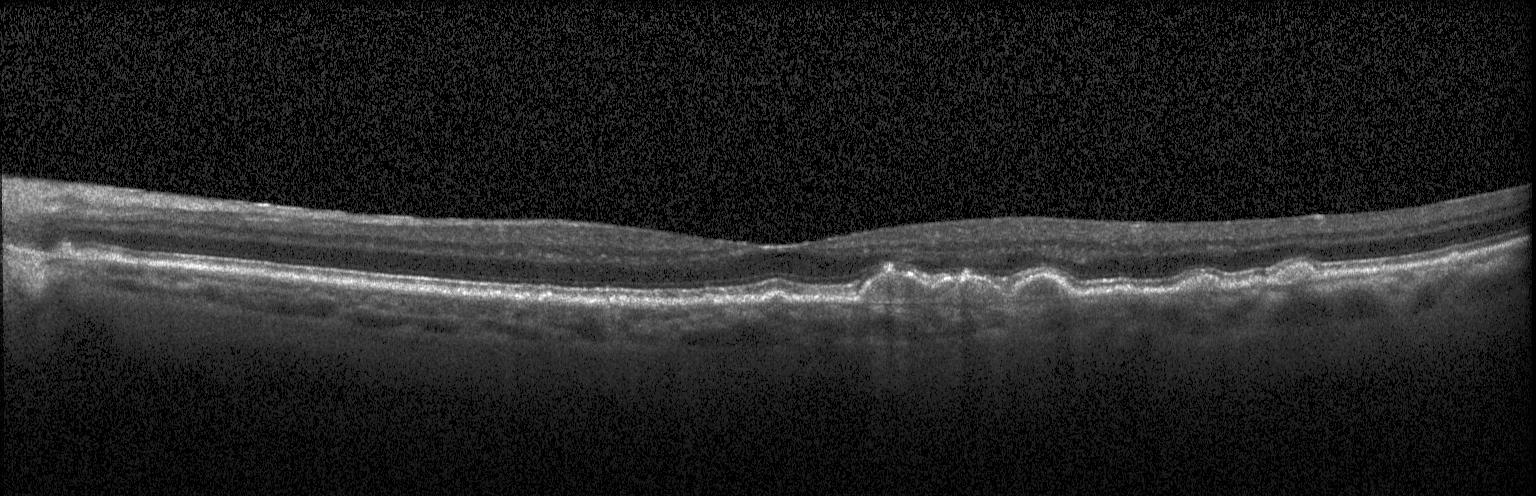 OCT line scan; Heidelberg Spectralis. Impression: choroidal neovascularization (CNV).